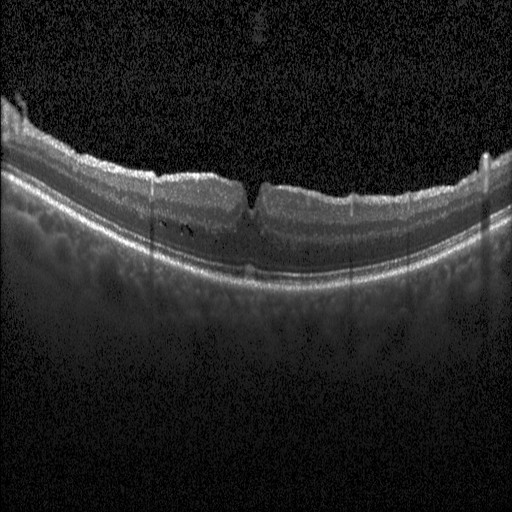
Spectral-domain OCT B-scan: diabetic macular edema (DME).